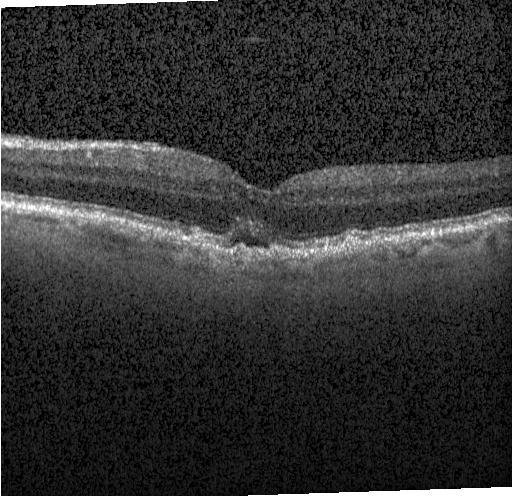
OCT finding: choroidal neovascularization (CNV).